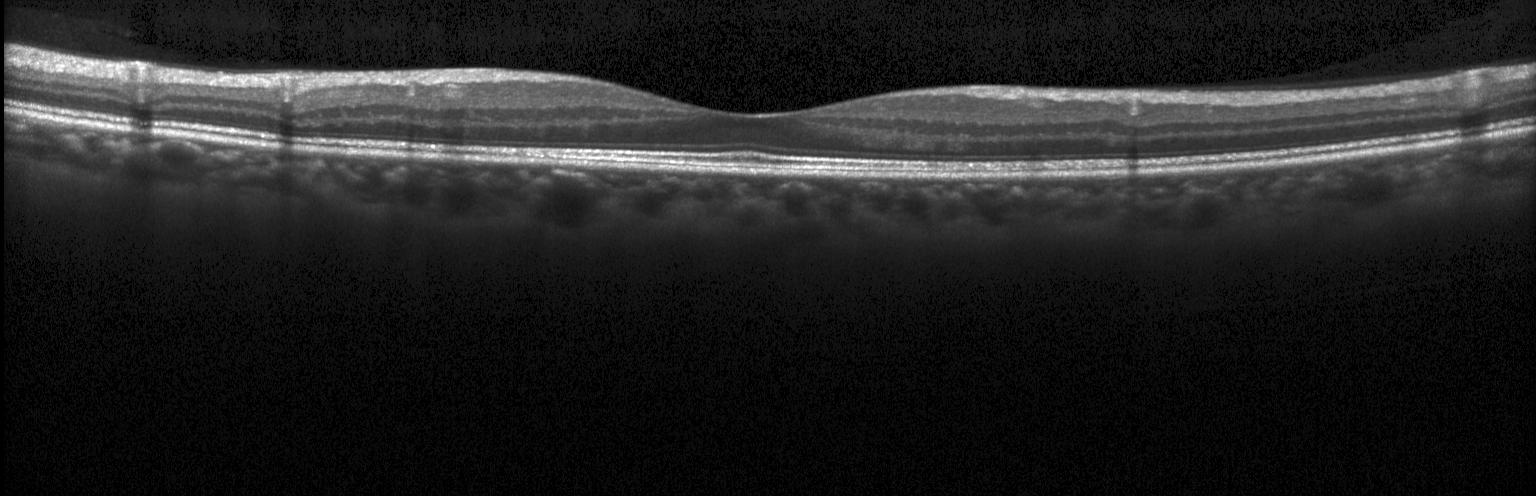 Finding: no choroidal neovascularization, no diabetic macular edema, and no drusen.